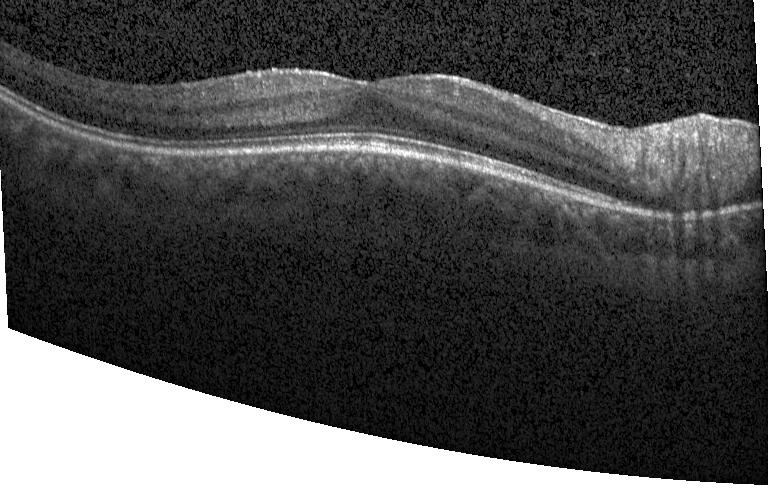

OCT line scan — The scan shows no CNV, DME, or drusen.